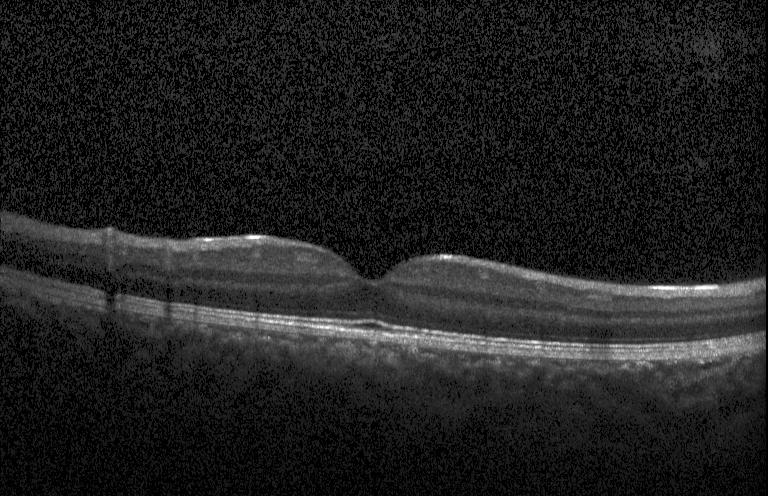
Finding: neither choroidal neovascularization, diabetic macular edema, nor drusen.